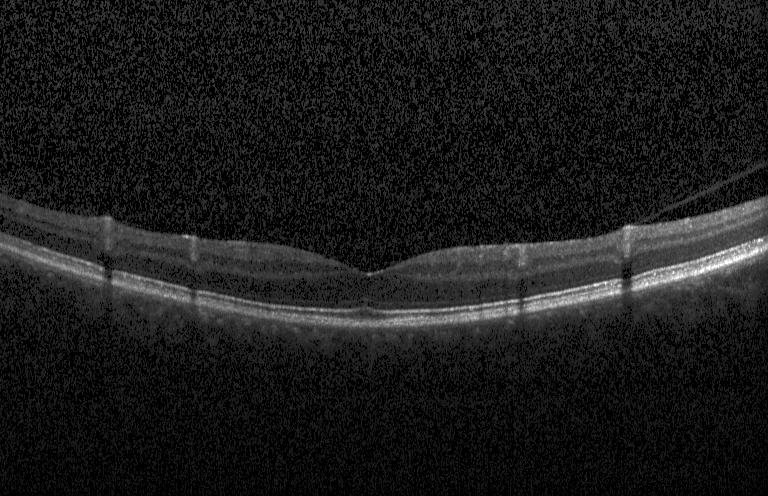

Optical coherence tomography scan — The scan shows neither choroidal neovascularization, diabetic macular edema, nor drusen.